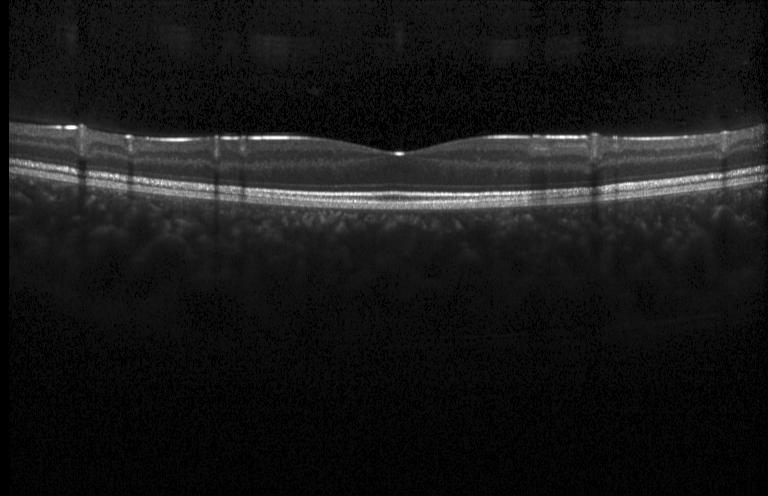

Heidelberg Spectralis OCT system, optical coherence tomography scan.
Dx: no evidence of CNV, DME, or drusen.